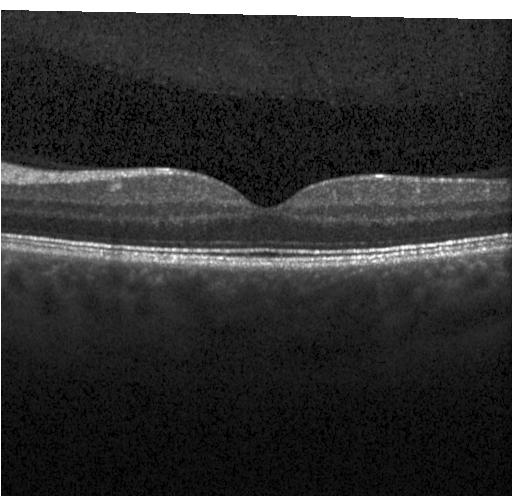

Dx: neither CNV, DME, nor drusen.